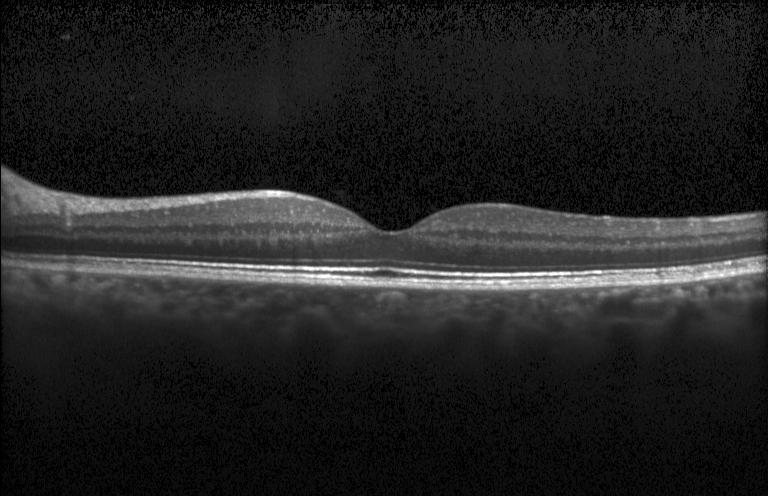 Retinal OCT cross-section showing no choroidal neovascularization, no diabetic macular edema, and no drusen.